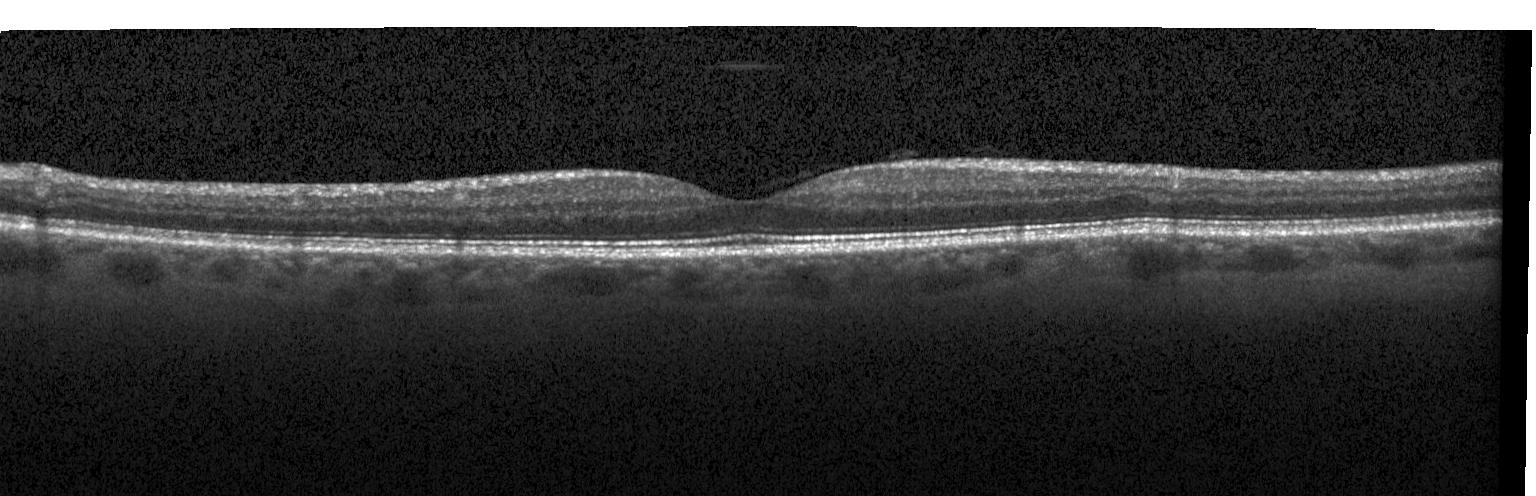

Fovea-centered · acquired on a Heidelberg Spectralis · OCT line scan — This B-scan demonstrates neither CNV, DME, nor drusen.